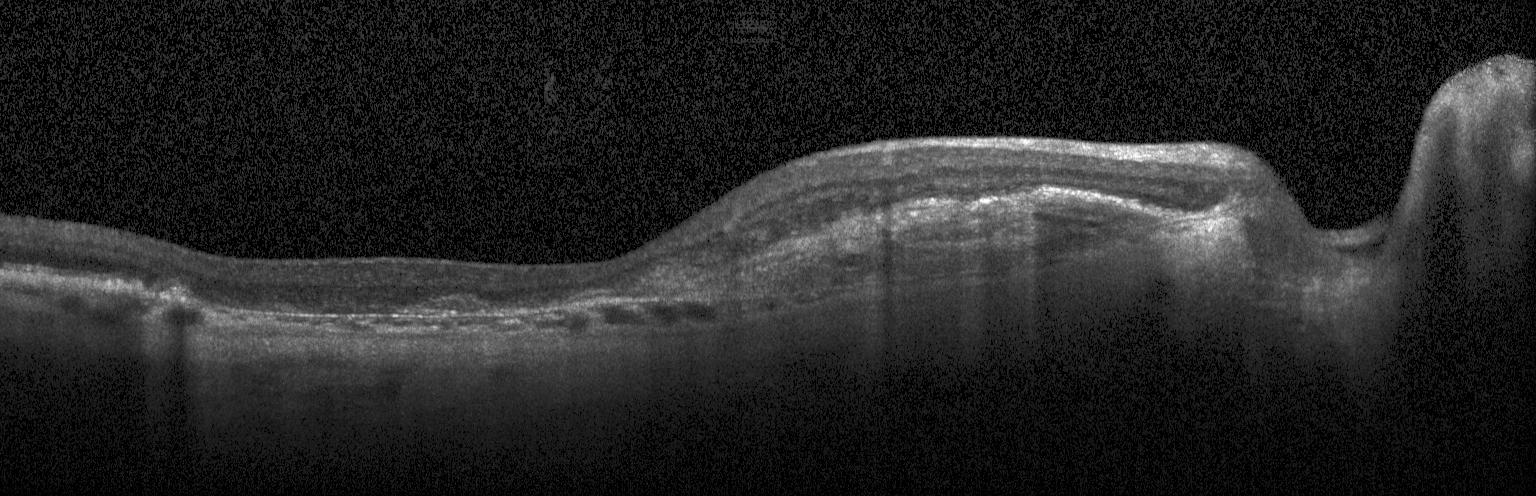
Retinal OCT cross-section.
A choroidal neovascular membrane.